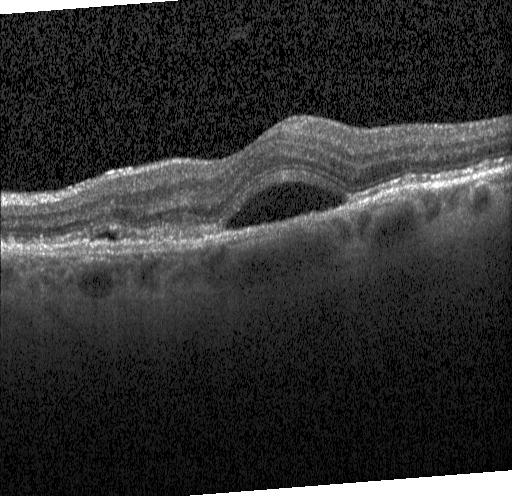
Diagnosis: choroidal neovascularization.